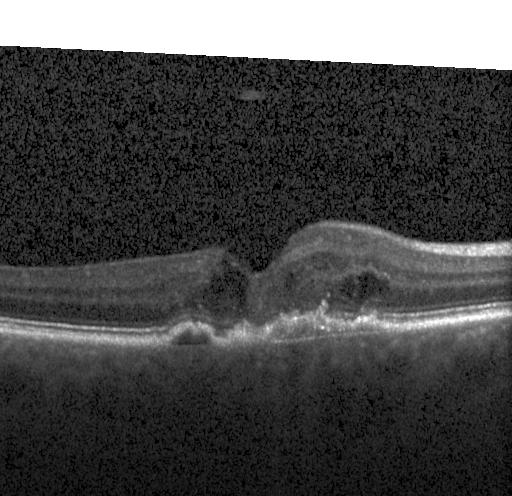
Optical coherence tomography B-scan · Heidelberg Spectralis OCT system.
Diagnosis: choroidal neovascularization (CNV).